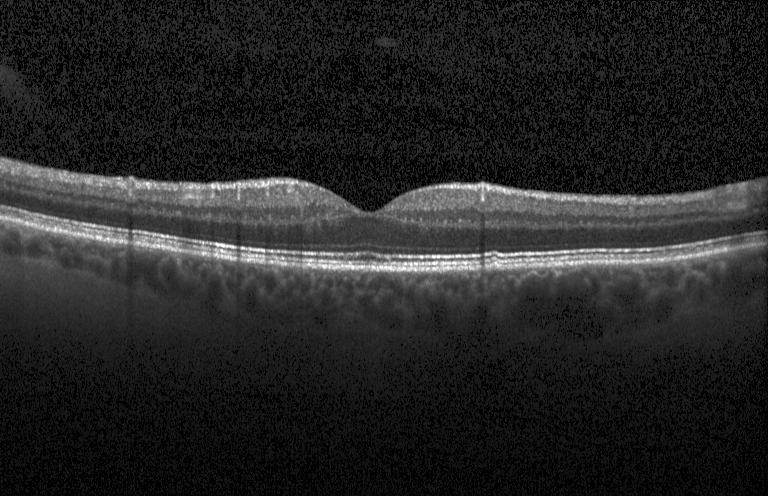

Impression: neither CNV, DME, nor drusen.